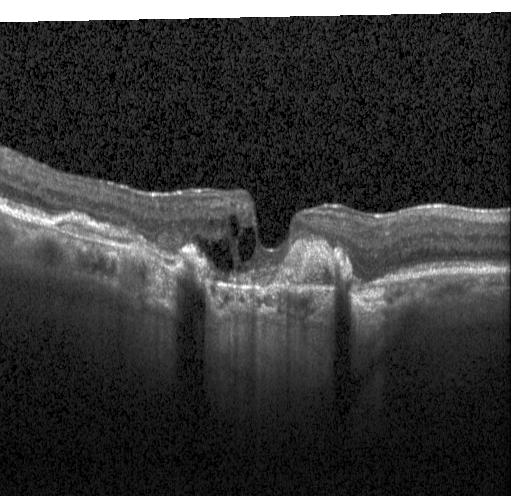
Horizontal scan through the fovea. Retinal OCT B-scan. Diagnosis: choroidal neovascularization (CNV).